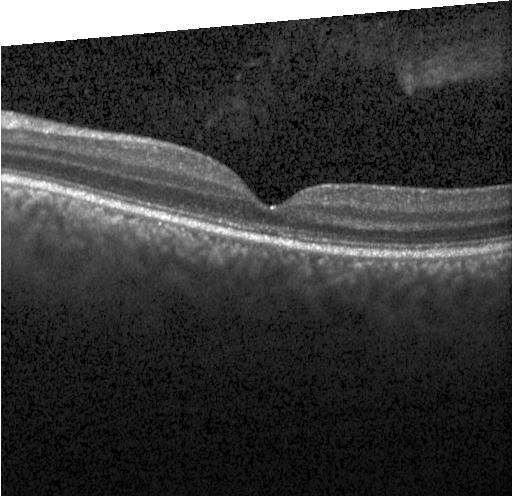

Macular OCT demonstrating neither CNV, DME, nor drusen.